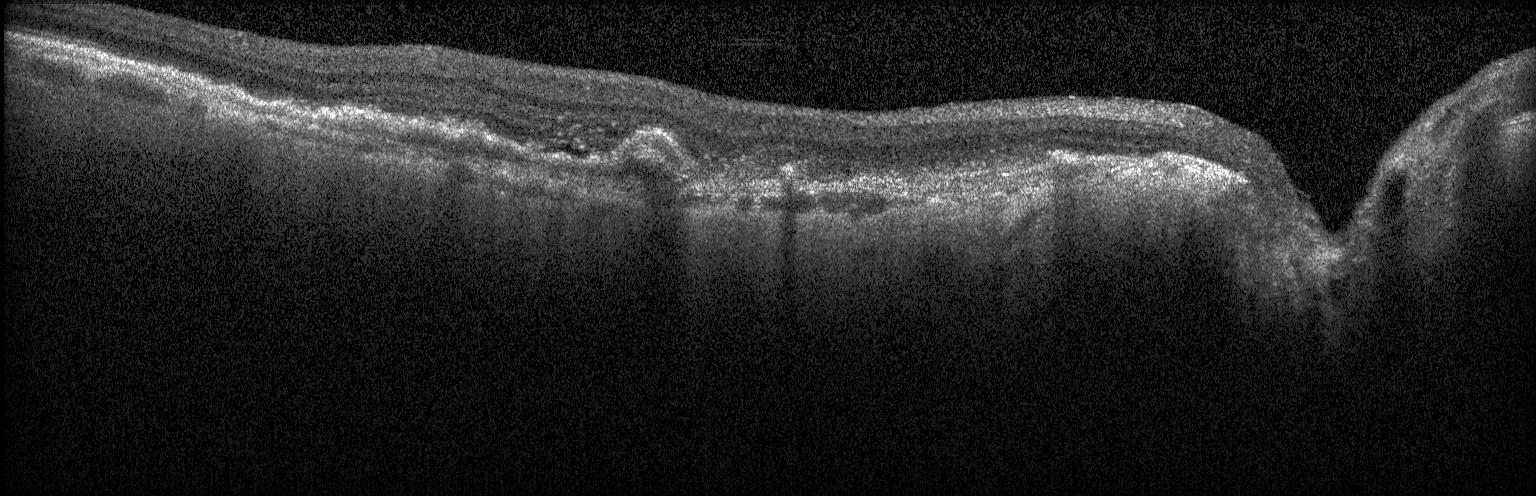 Dx: choroidal neovascularization.